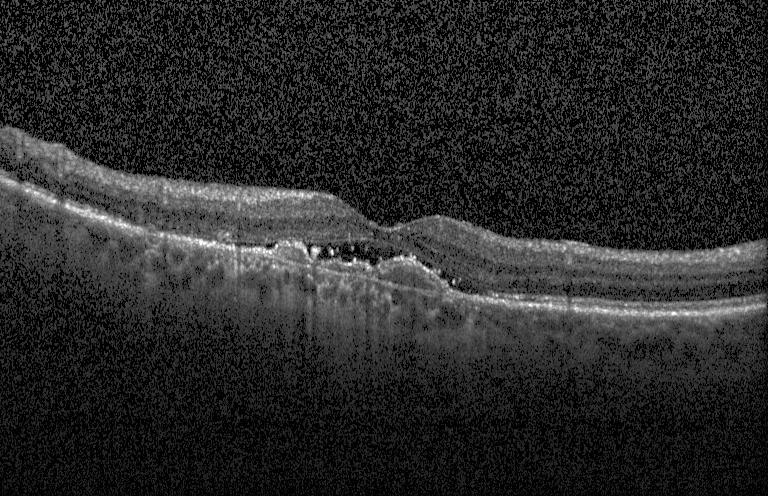
Impression: choroidal neovascularization (CNV).